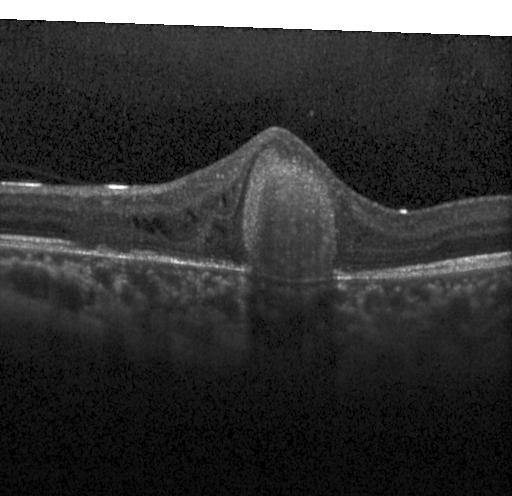 OCT B-scan showing choroidal neovascularization.